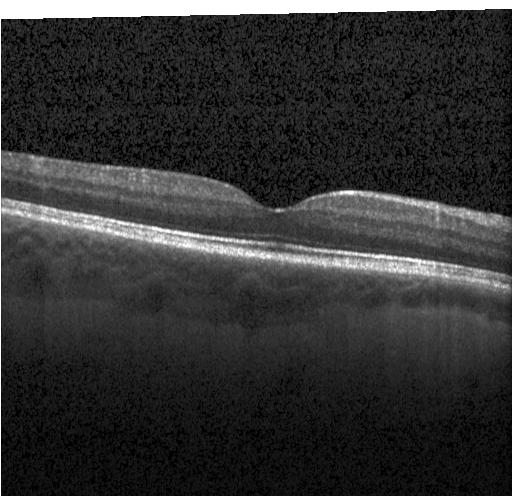 OCT B-scan; spectral-domain OCT; macular scan
Finding: no evidence of CNV, DME, or drusen.